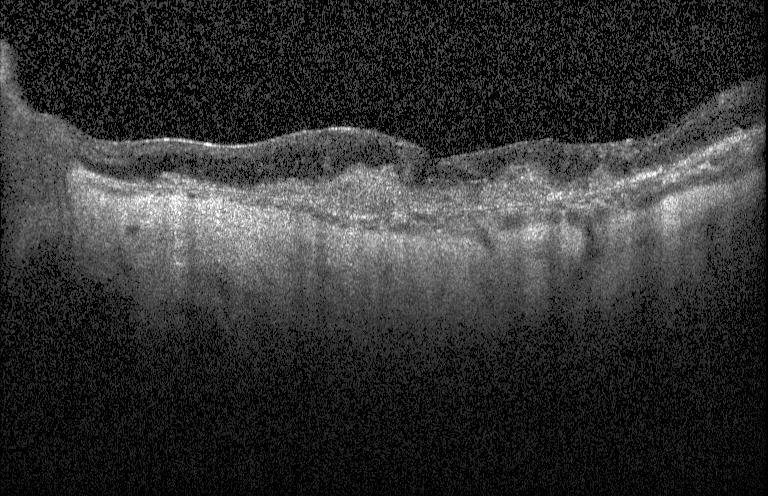 Impression: CNV.